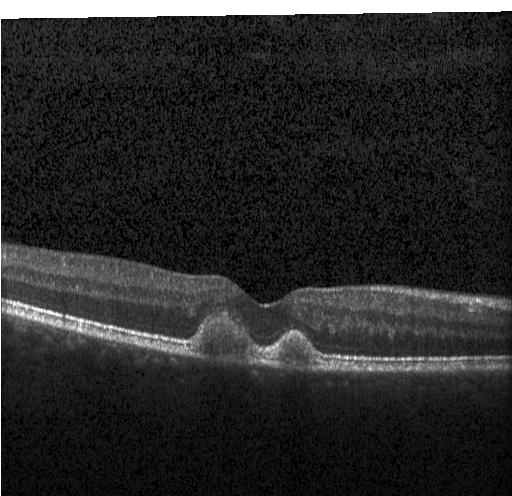 Assessment: multiple drusen.